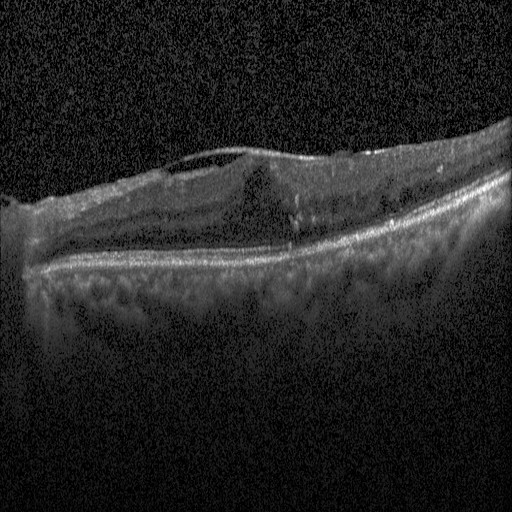 Centered on the fovea · optical coherence tomography scan. Diabetic macular edema (DME).